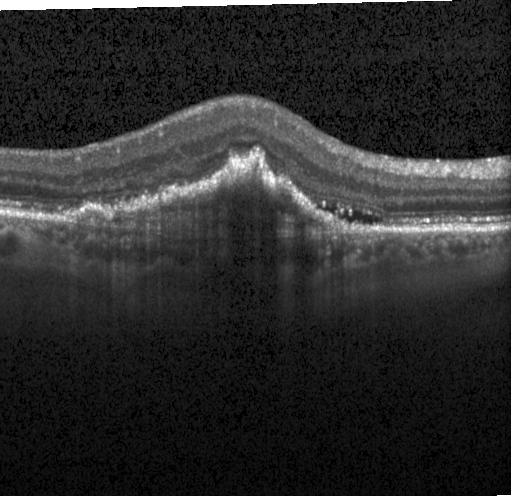
Finding: a choroidal neovascular membrane.